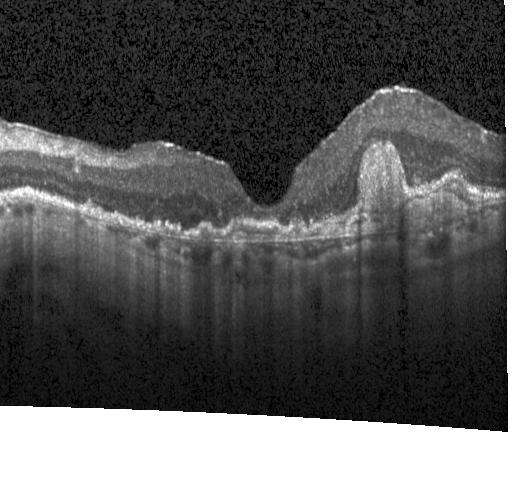 Through the macula · Heidelberg Spectralis · OCT line scan · SD-OCT.
Assessment: a choroidal neovascular membrane.